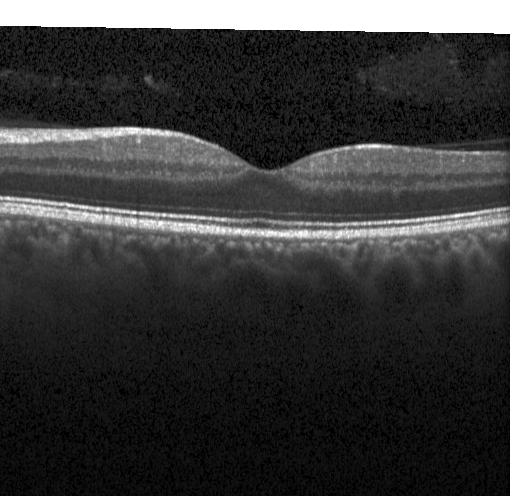
Macular OCT: no choroidal neovascularization, no diabetic macular edema, and no drusen.